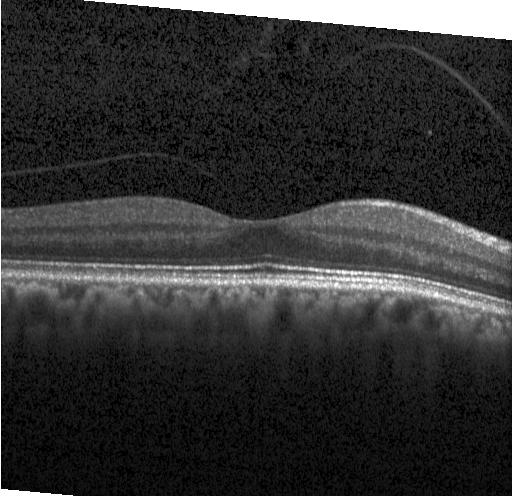 OCT scan showing no choroidal neovascularization, no diabetic macular edema, and no drusen.